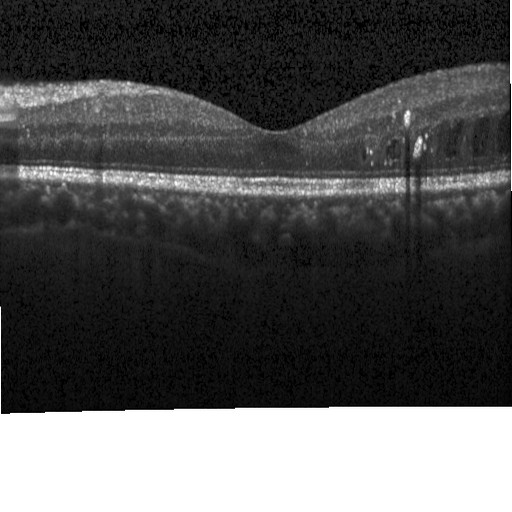 Finding: diabetic macular edema (DME).